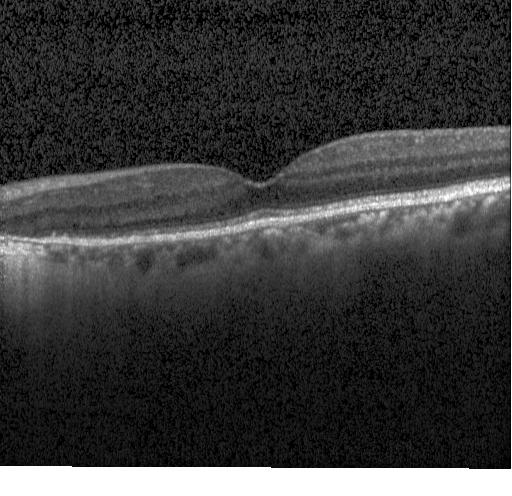 Macular scan. Optical coherence tomography B-scan. Heidelberg Spectralis. SD-OCT. The scan shows no choroidal neovascularization, no diabetic macular edema, and no drusen.